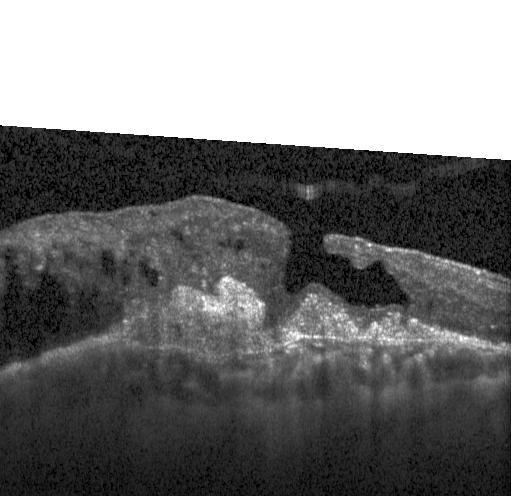

SD-OCT; Heidelberg Spectralis; OCT line scan.
OCT finding: choroidal neovascularization (CNV).